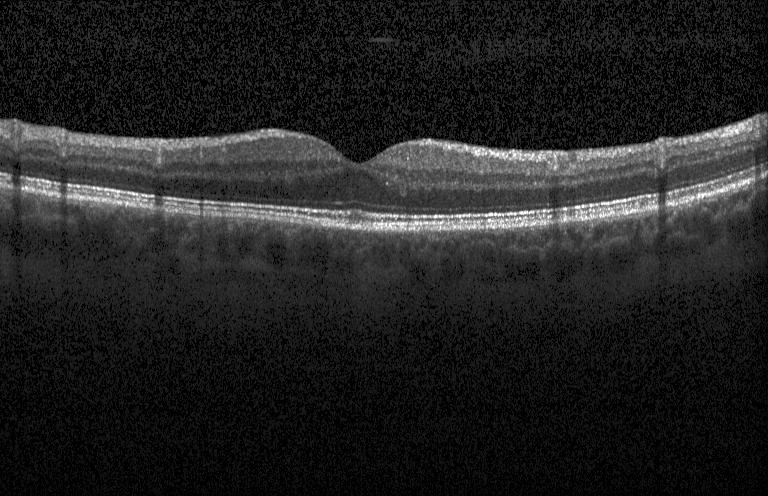 Through the macula. Heidelberg Spectralis. Optical coherence tomography B-scan
The scan shows no evidence of choroidal neovascularization, diabetic macular edema, or drusen.